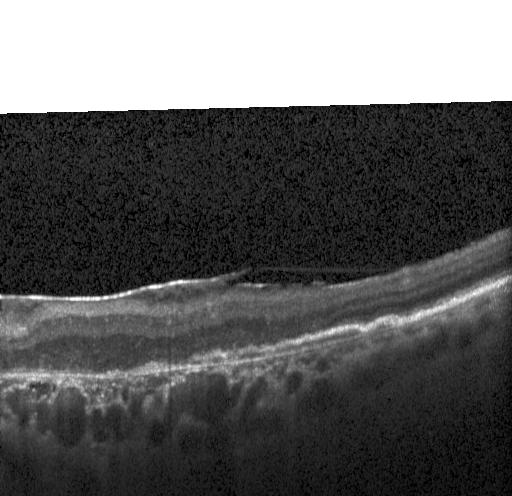 Optical coherence tomography B-scan, Heidelberg Spectralis, SD-OCT — Finding: a choroidal neovascular membrane.